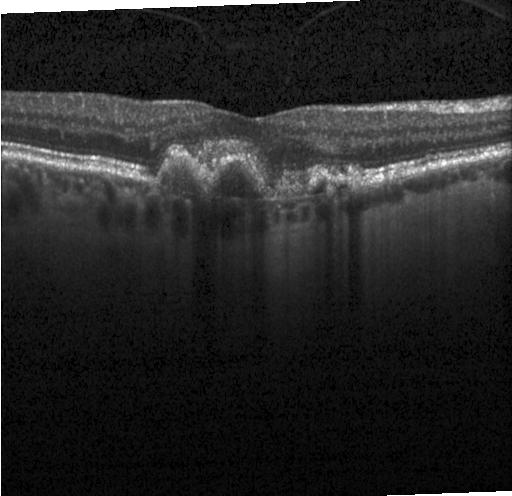

Optical coherence tomography scan · horizontal scan through the fovea. This B-scan demonstrates choroidal neovascularization (CNV).